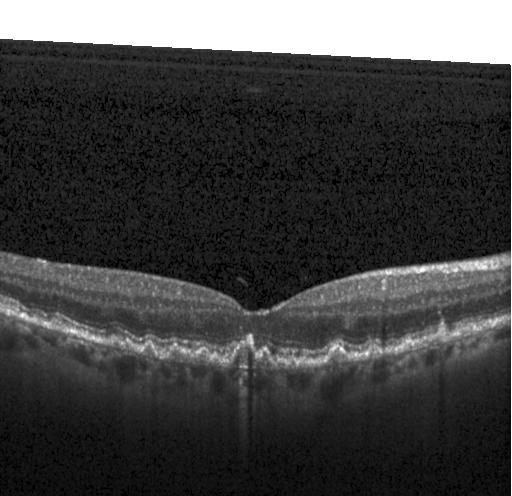 Finding: drusen.